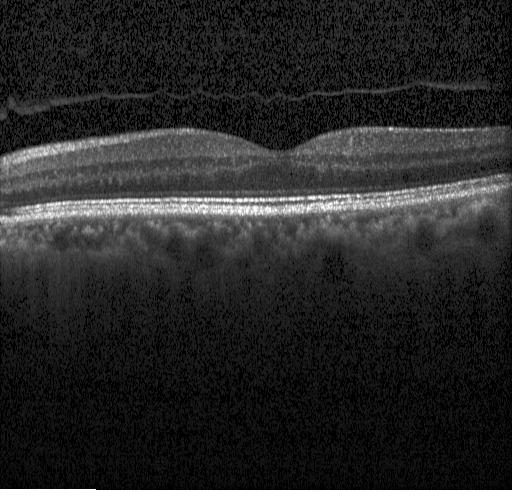
Impression: neither choroidal neovascularization, diabetic macular edema, nor drusen.